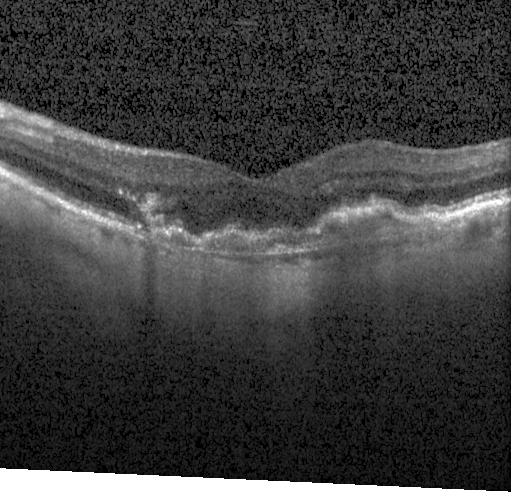

Diagnosis: a choroidal neovascular membrane.